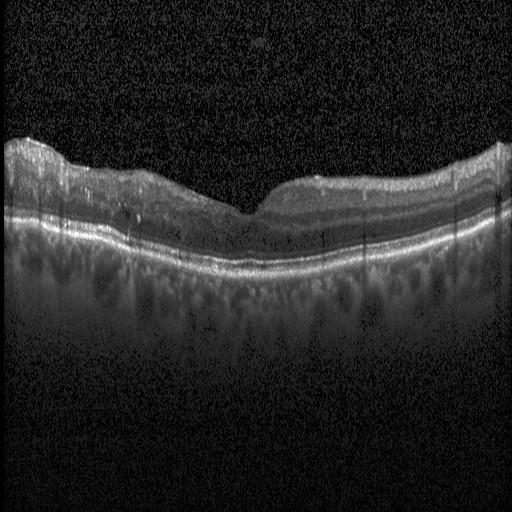
Spectral-domain OCT. Retinal OCT B-scan. Heidelberg Spectralis. Fovea-centered.
DME.